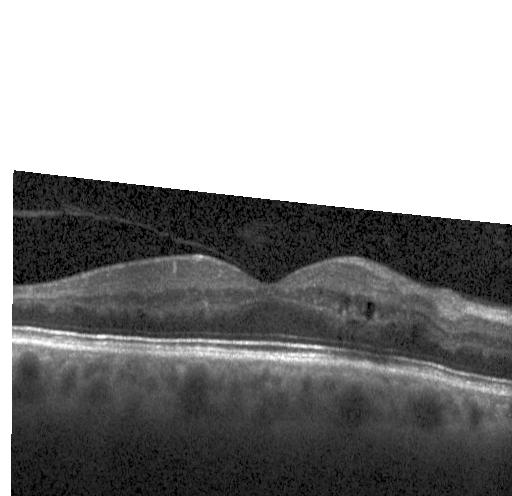

Spectral-domain OCT, acquired on a Heidelberg Spectralis, optical coherence tomography scan, centered on the fovea.
Finding: DME.